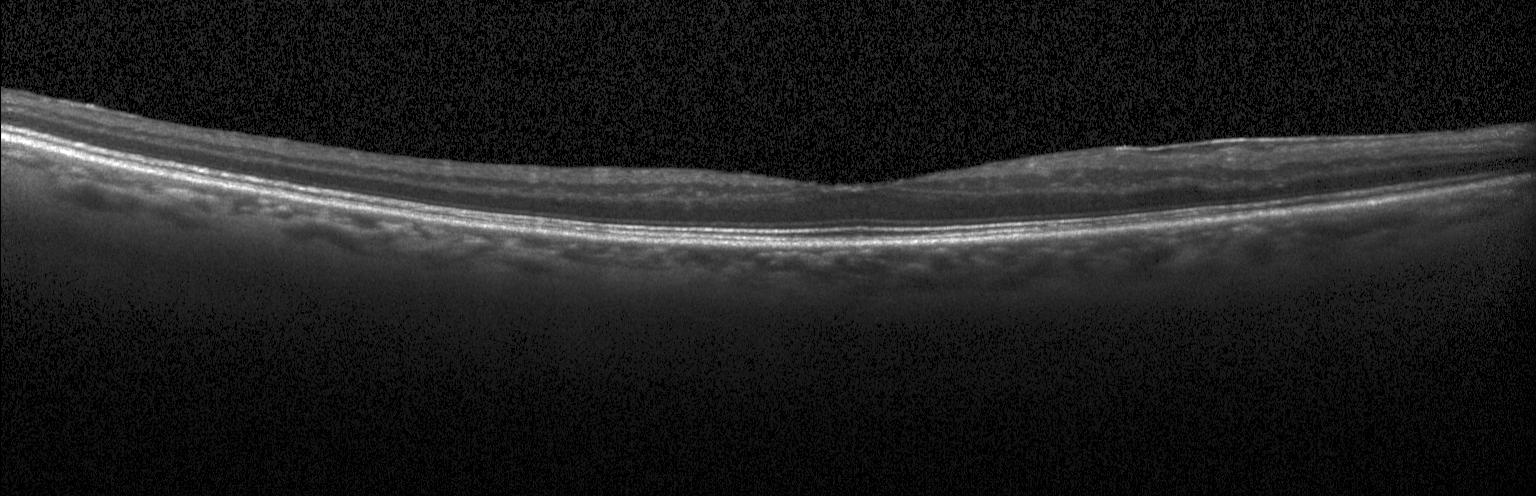
OCT line scan.
No choroidal neovascularization, diabetic macular edema, or drusen.